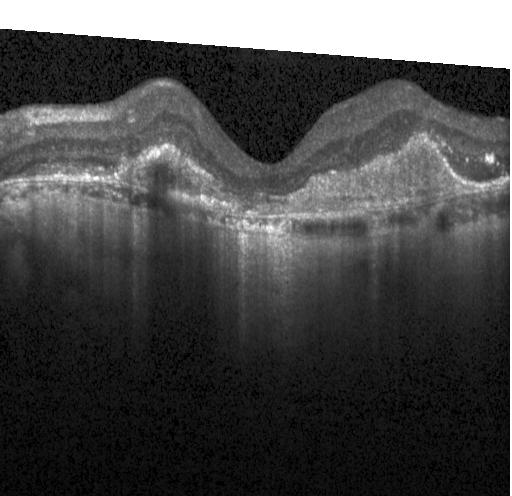 Diagnosis: a choroidal neovascular membrane.